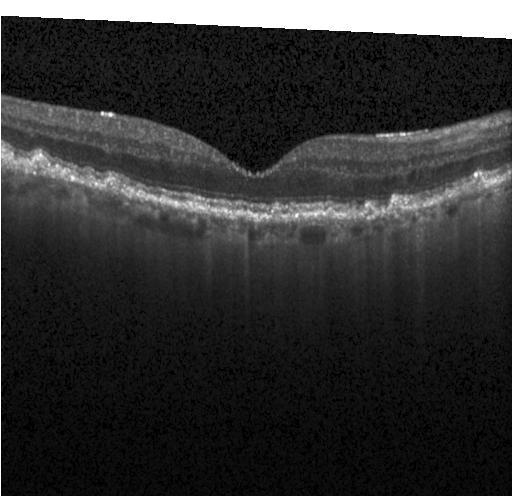
Macular OCT: drusen.